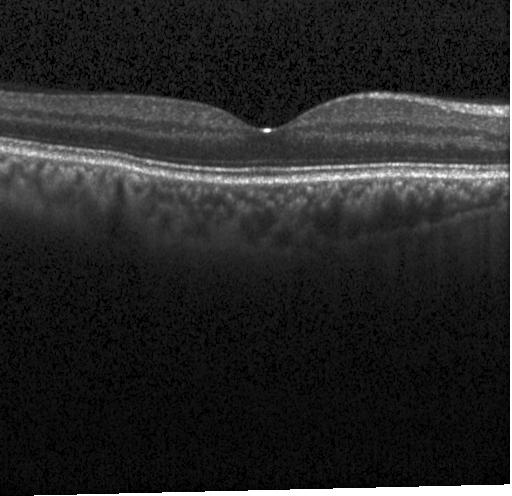
The scan shows no evidence of choroidal neovascularization, diabetic macular edema, or drusen.